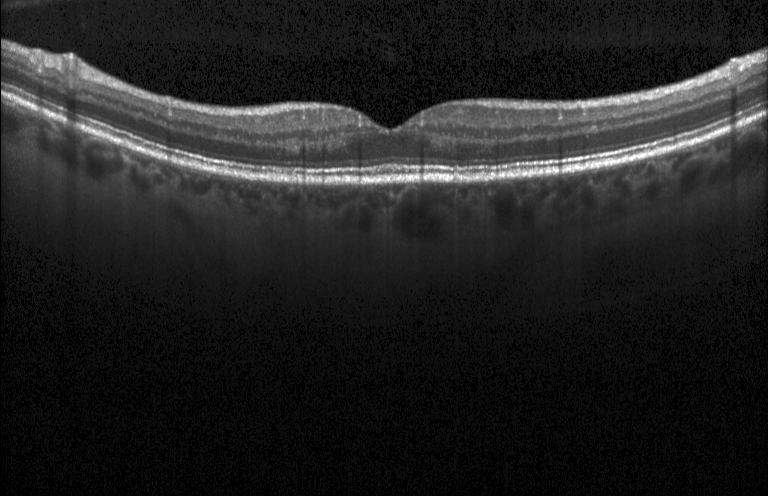 Heidelberg Spectralis OCT system. Through the macula. Optical coherence tomography B-scan. No evidence of choroidal neovascularization, diabetic macular edema, or drusen.